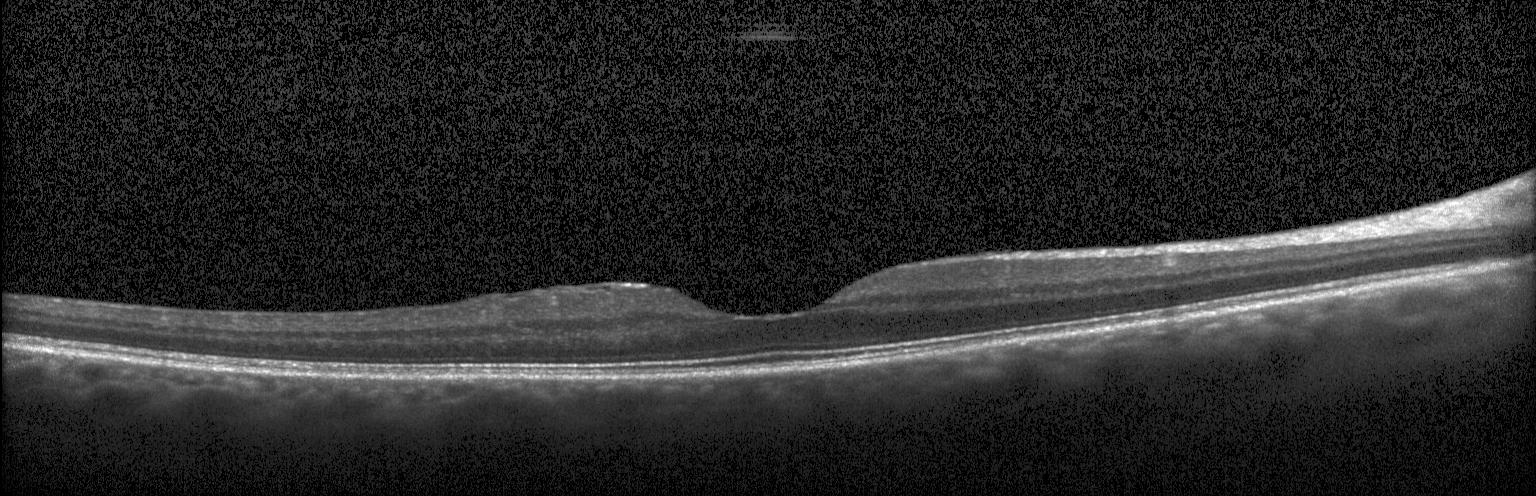
OCT line scan; acquired on a Heidelberg Spectralis; horizontal scan through the fovea — OCT finding: no choroidal neovascularization, diabetic macular edema, or drusen.